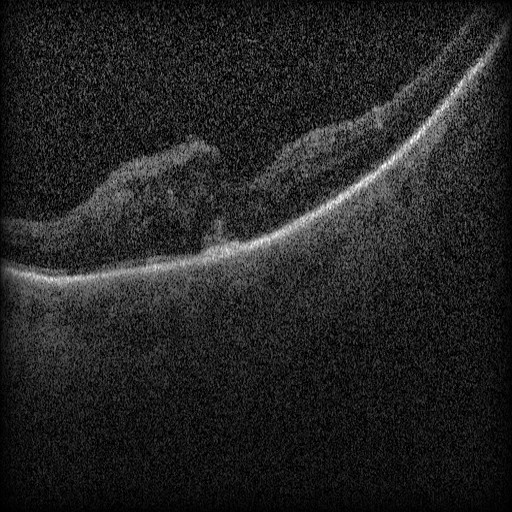
Heidelberg Spectralis; optical coherence tomography scan
Assessment: diabetic macular edema.